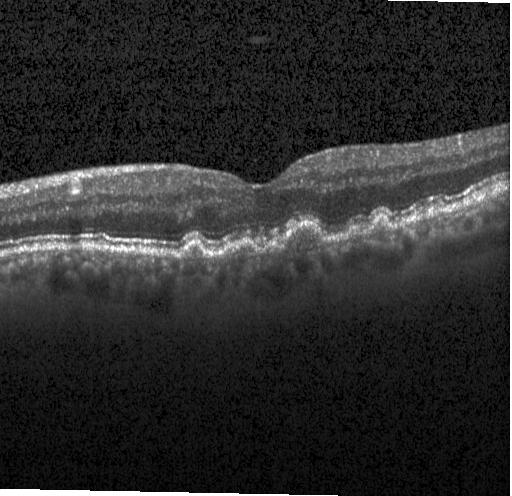

OCT B-scan. Heidelberg Spectralis OCT system. SD-OCT
Impression: multiple drusen.